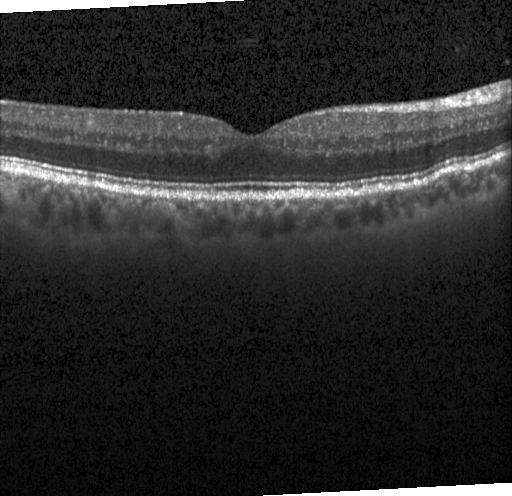

Spectral-domain OCT. Through the macula. Optical coherence tomography B-scan
The scan shows neither choroidal neovascularization, diabetic macular edema, nor drusen.